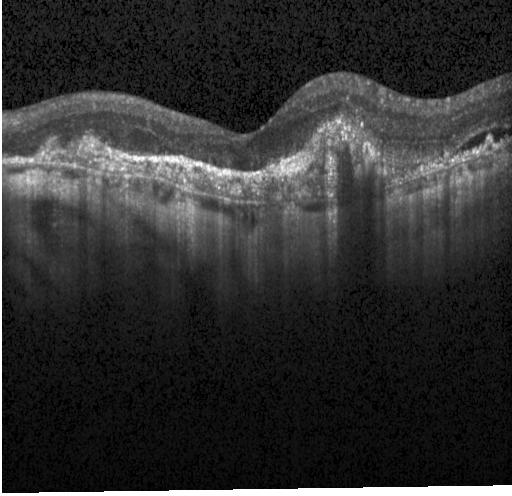 Optical coherence tomography scan, centered on the fovea, spectral-domain optical coherence tomography, Heidelberg Spectralis. Impression: CNV.